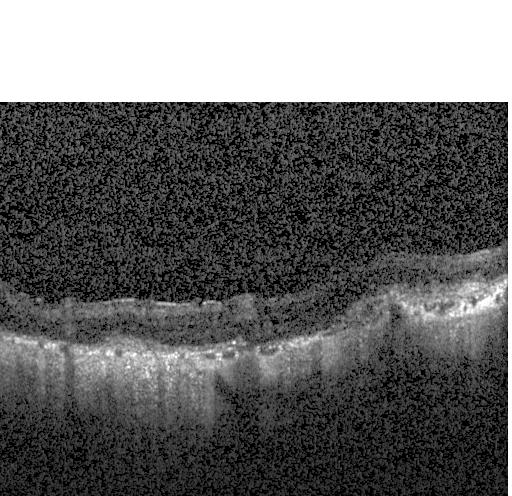 Impression: CNV.